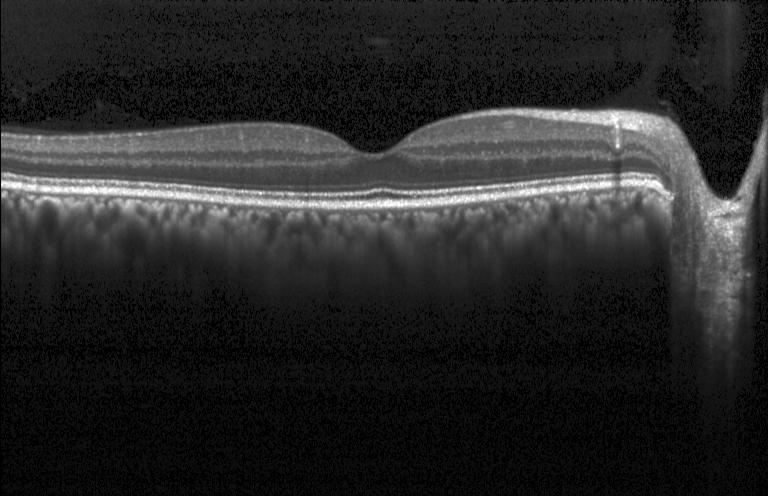 OCT B-scan · SD-OCT
This B-scan demonstrates no choroidal neovascularization, diabetic macular edema, or drusen.